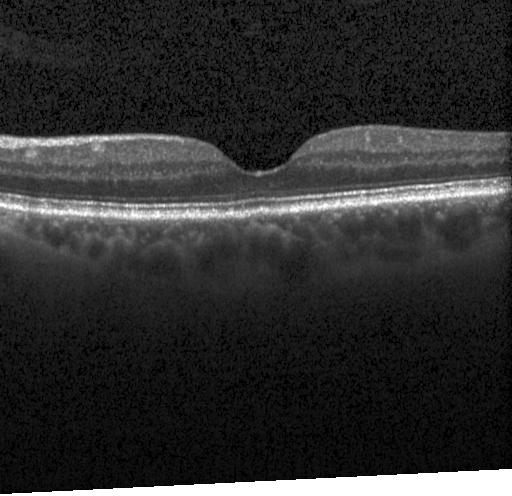

Optical coherence tomography scan — Diagnosis: no evidence of CNV, DME, or drusen.